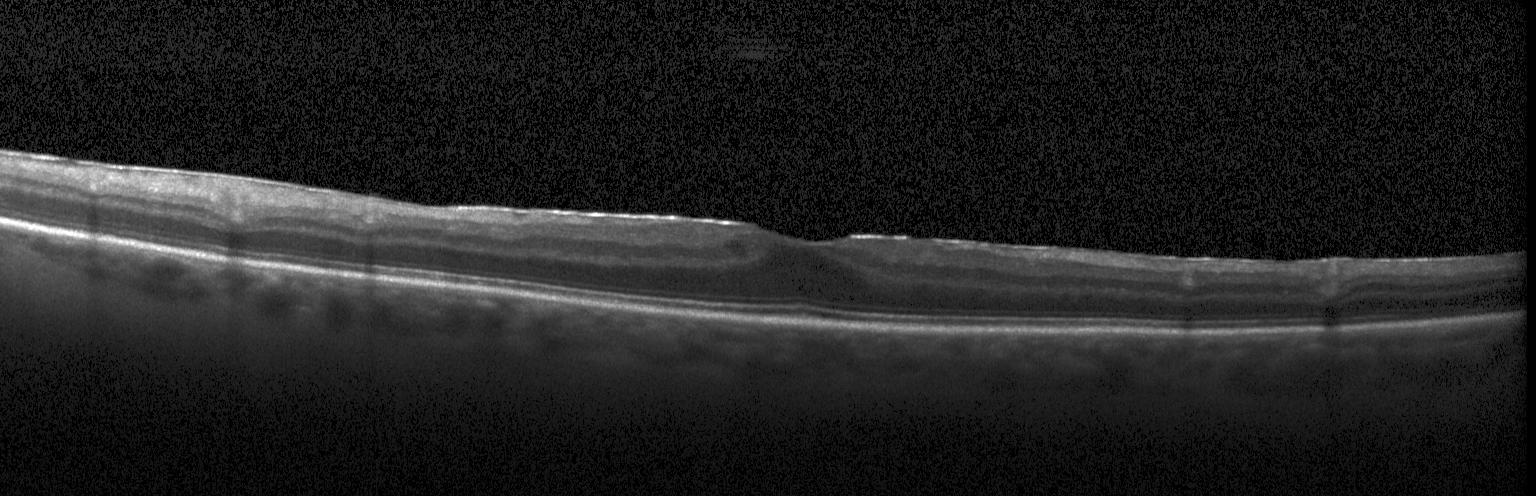 Fovea-centered, instrument: Heidelberg Spectralis, OCT B-scan, spectral-domain optical coherence tomography.
Diagnosis: DME.